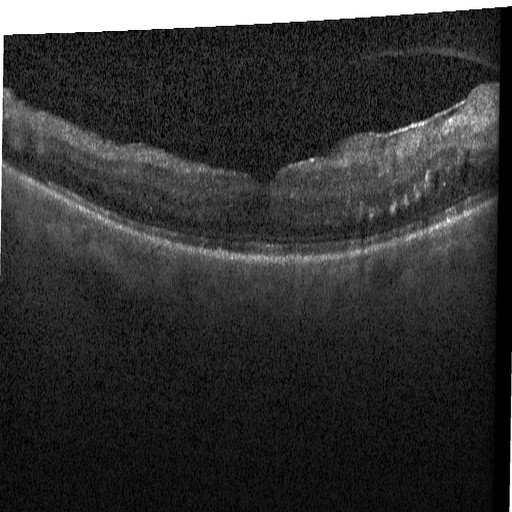 Centered on the fovea · retinal OCT B-scan · acquired on a Heidelberg Spectralis. Diagnosis: diabetic macular edema (DME).